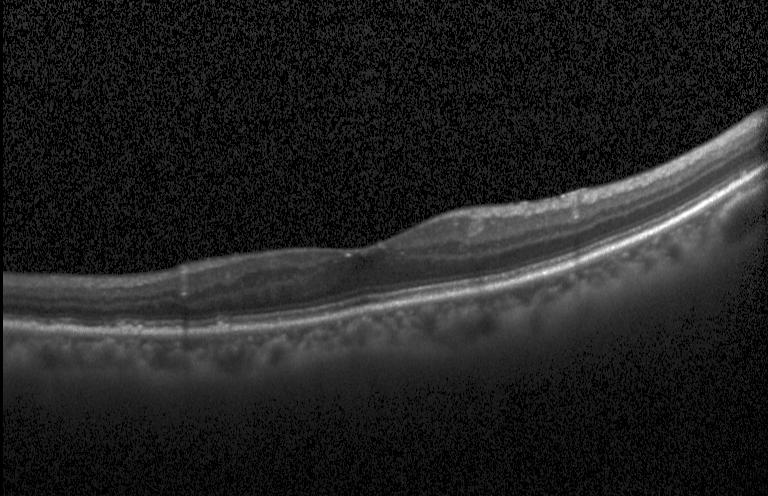
Finding: sub-RPE drusenoid deposits.